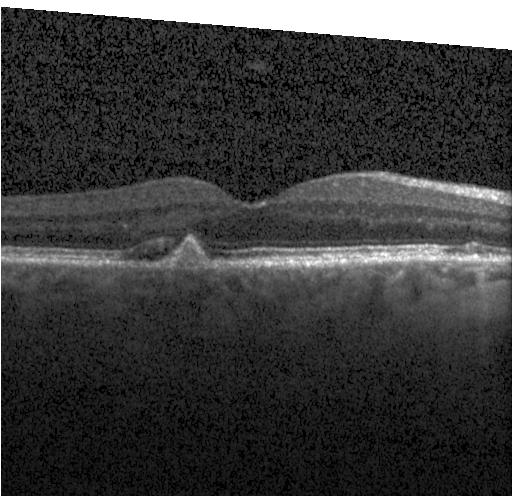

Macular OCT demonstrating choroidal neovascularization (CNV).